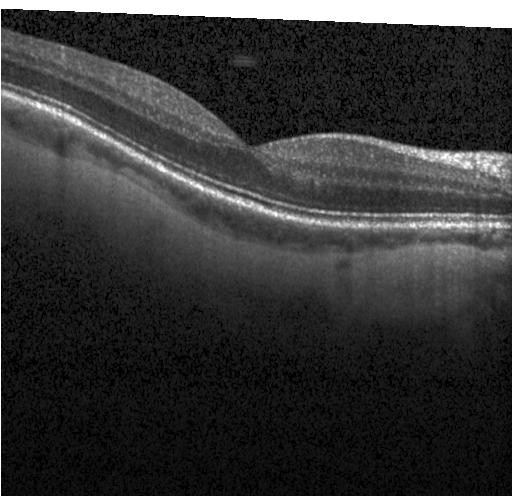 Through the macula · retinal OCT B-scan · spectral-domain OCT. Macular OCT: no CNV, DME, or drusen.